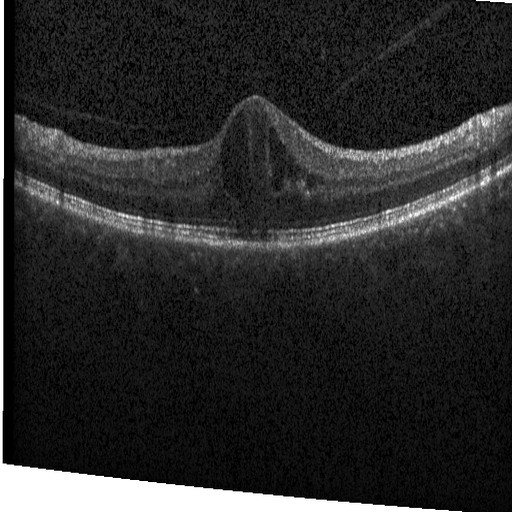 Heidelberg Spectralis OCT system; optical coherence tomography B-scan
The scan shows diabetic macular edema (DME).